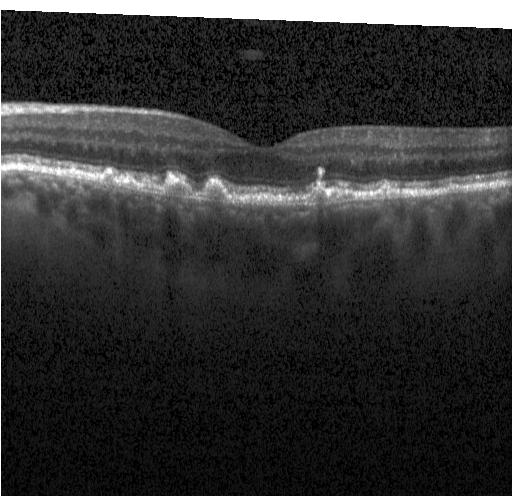
Retinal OCT cross-section, fovea-centered. Assessment: multiple drusen.